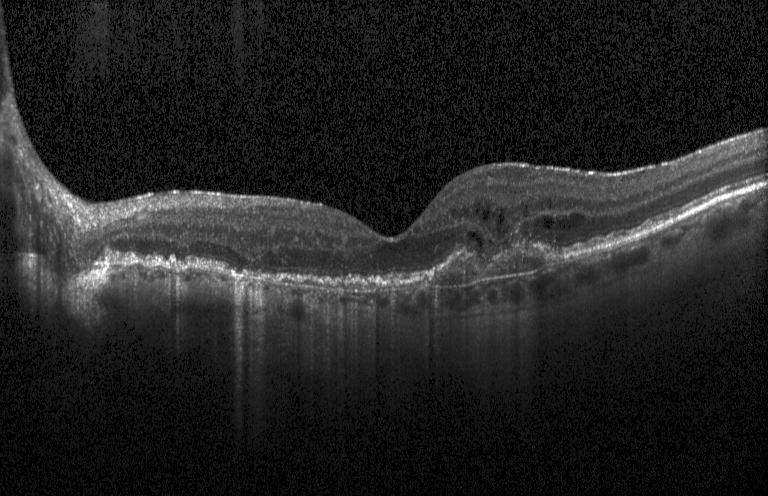
Instrument: Heidelberg Spectralis; optical coherence tomography scan; centered on the fovea; spectral-domain optical coherence tomography
Assessment: CNV.